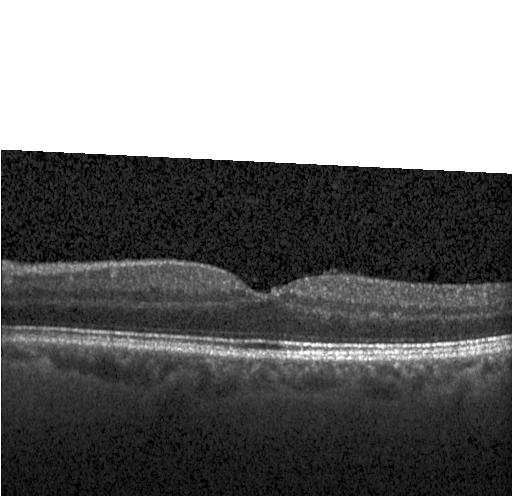

Retinal OCT B-scan, spectral-domain OCT, Heidelberg Spectralis — Finding: no evidence of CNV, DME, or drusen.